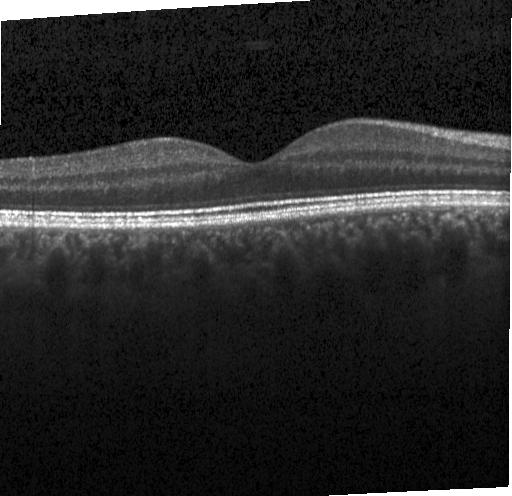
OCT B-scan · Heidelberg Spectralis OCT system · through the macula · spectral-domain optical coherence tomography
Diagnosis: no choroidal neovascularization, diabetic macular edema, or drusen.